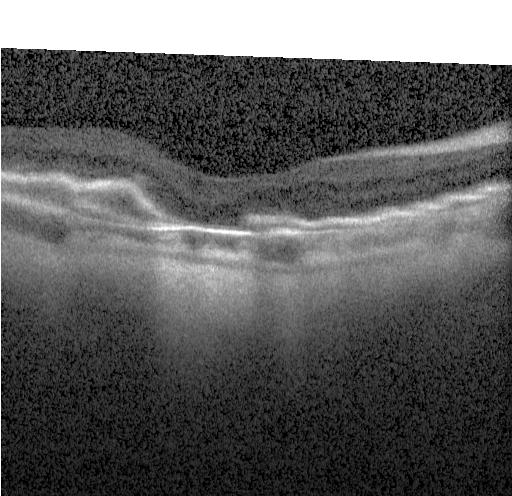
Finding: a choroidal neovascular membrane.